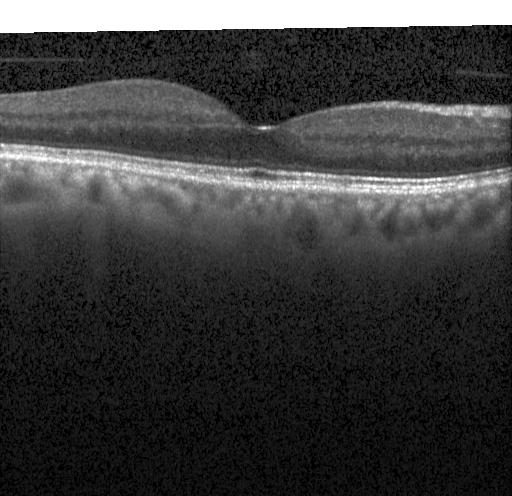
Through the macula. Heidelberg Spectralis OCT system. Spectral-domain optical coherence tomography. Retinal OCT B-scan. Diagnosis: no choroidal neovascularization, diabetic macular edema, or drusen.